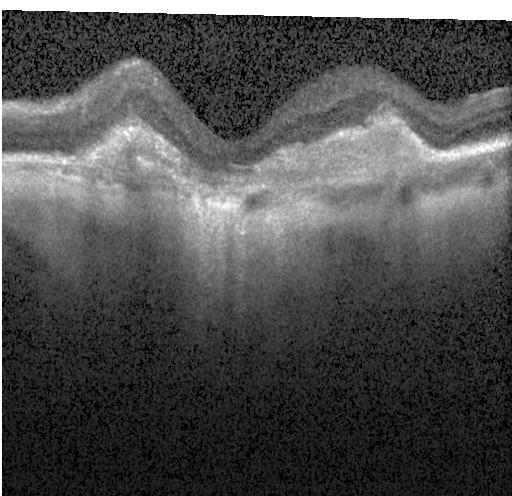
Heidelberg Spectralis; OCT line scan. Impression: choroidal neovascularization.